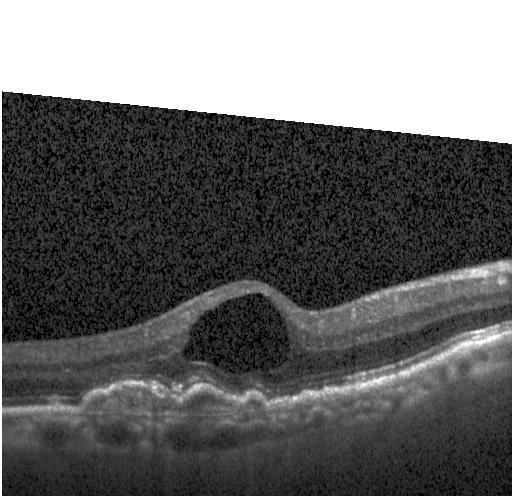 OCT line scan.
Finding: a choroidal neovascular membrane.